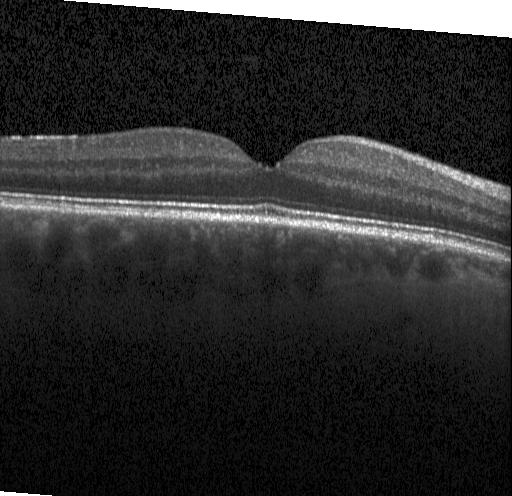

OCT finding: no evidence of choroidal neovascularization, diabetic macular edema, or drusen.